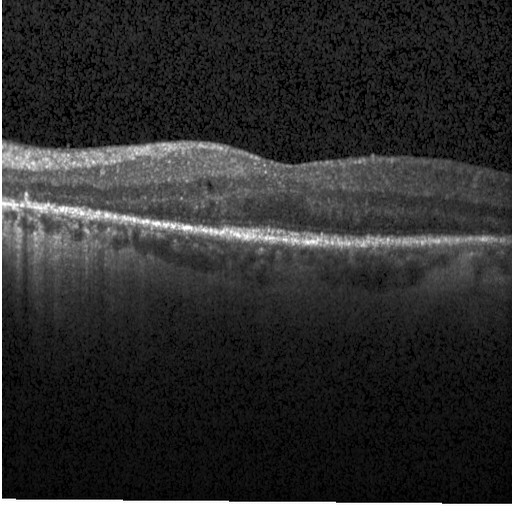 DME.